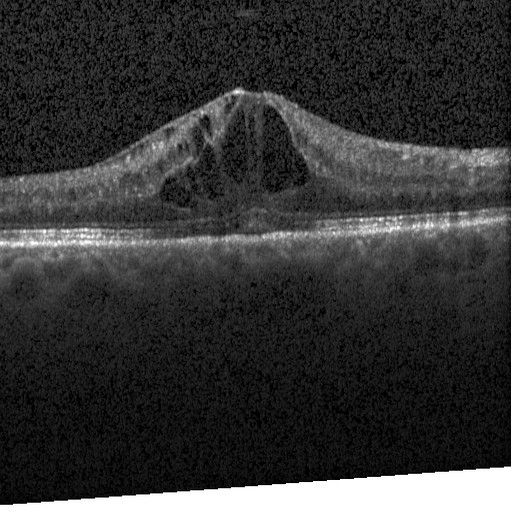
OCT line scan
Dx: diabetic macular edema (DME).